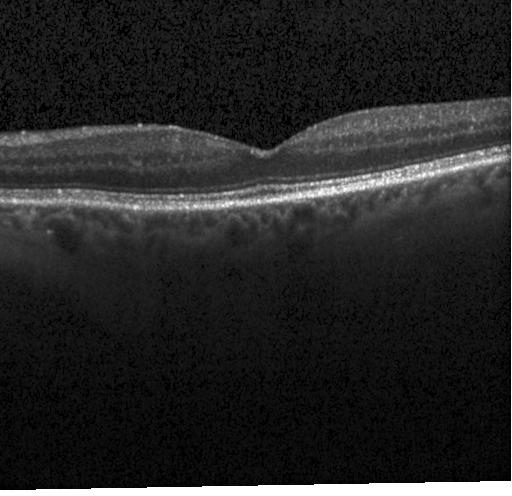

Finding: no evidence of choroidal neovascularization, diabetic macular edema, or drusen.